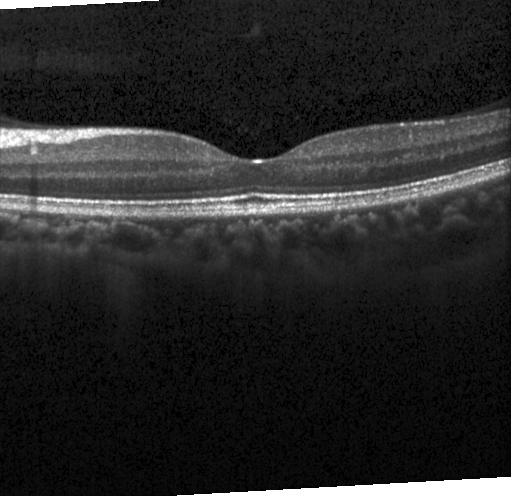
Fovea-centered; OCT line scan — Impression: no choroidal neovascularization, no diabetic macular edema, and no drusen.